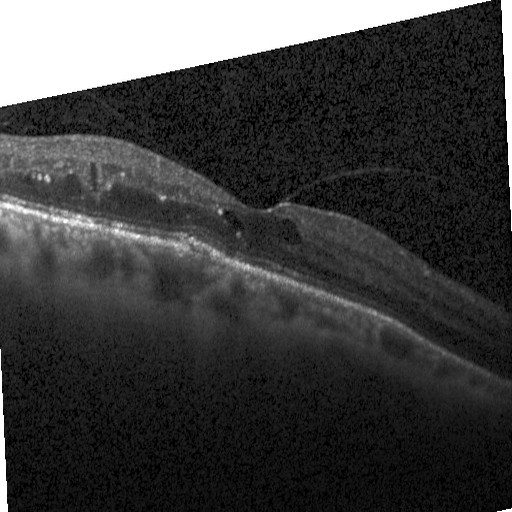 Optical coherence tomography scan
Diagnosis: diabetic macular edema (DME).